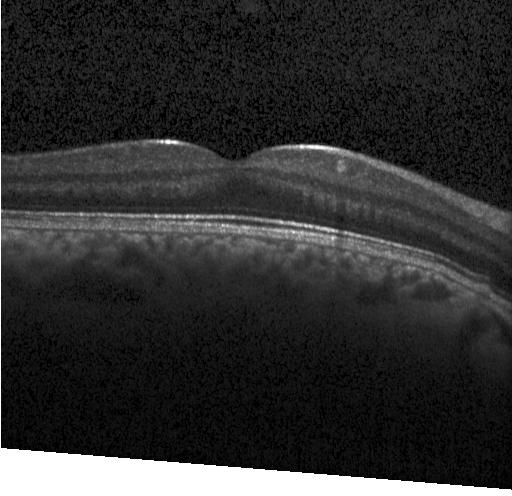 Diagnosis: neither choroidal neovascularization, diabetic macular edema, nor drusen.